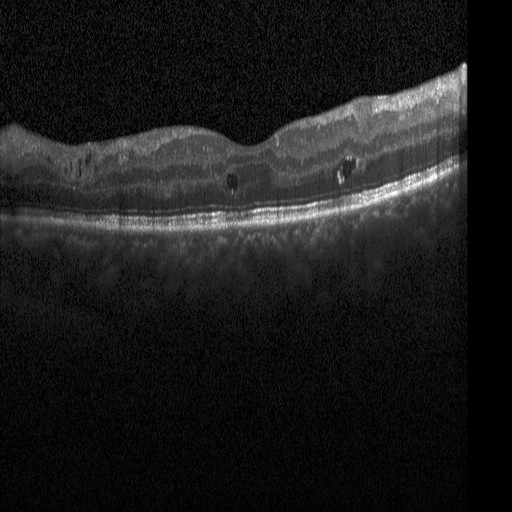

Macular OCT: diabetic macular edema.